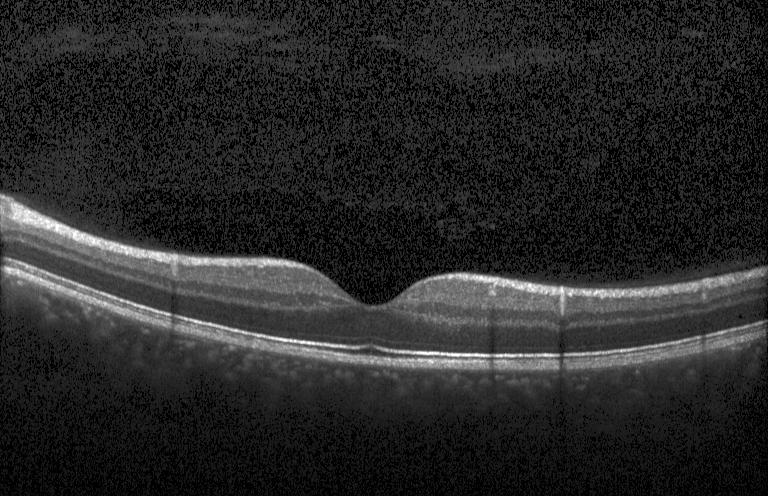
Assessment: no evidence of choroidal neovascularization, diabetic macular edema, or drusen.